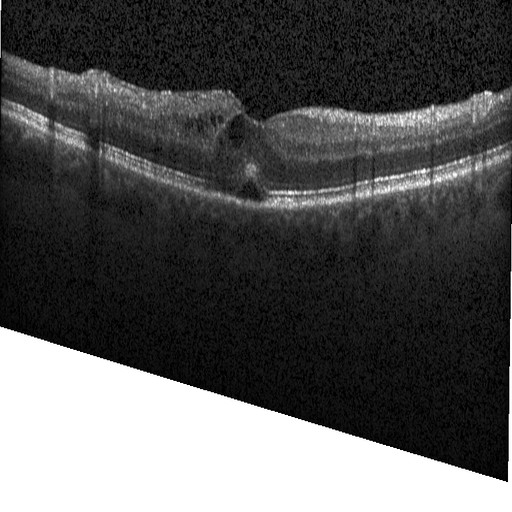 Through the macula. Heidelberg Spectralis OCT system. Spectral-domain optical coherence tomography. Optical coherence tomography scan
Diagnosis: diabetic macular edema.